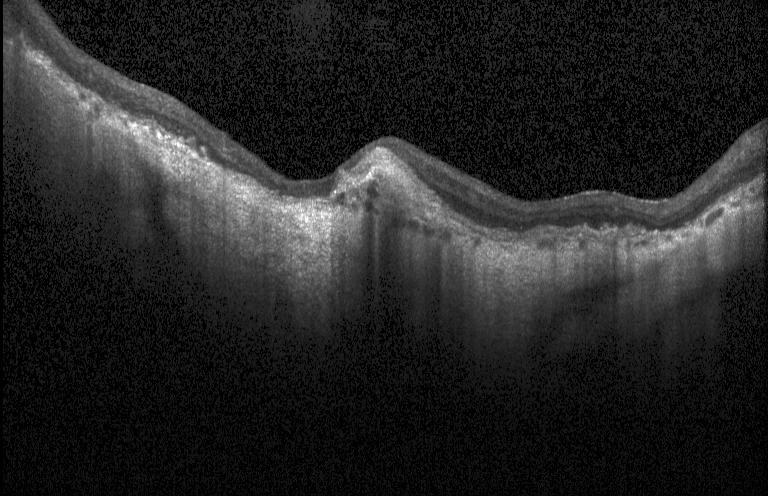

OCT line scan; macular scan.
This B-scan demonstrates a choroidal neovascular membrane.